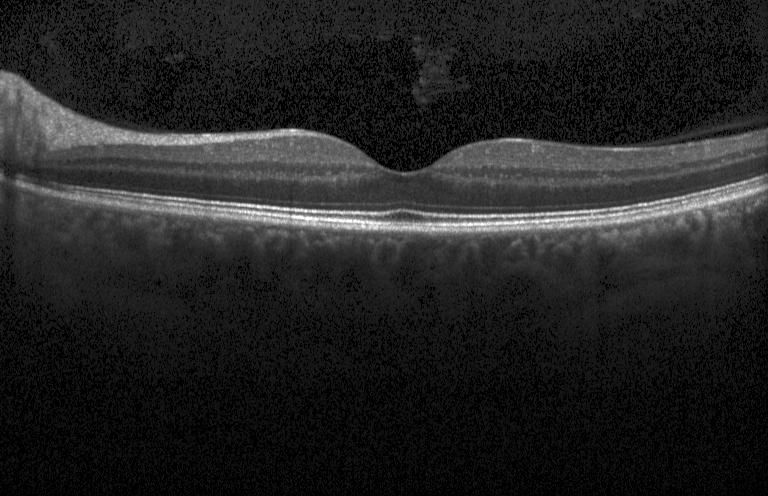 Macular OCT: no choroidal neovascularization, diabetic macular edema, or drusen.